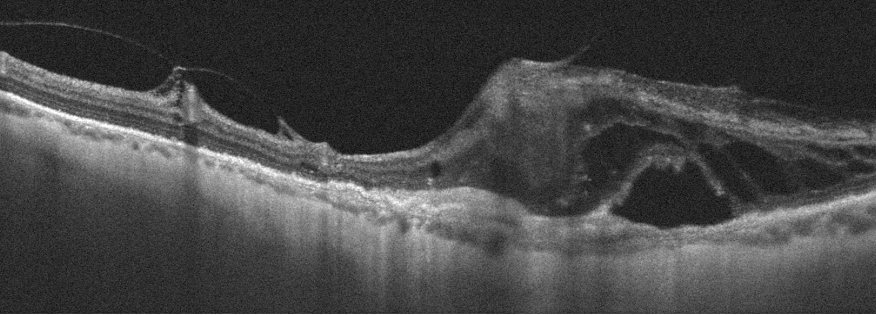
Retinal OCT cross-section; instrument: Optovue Avanti RTVue XR; through the macula. Finding: age-related macular degeneration (AMD).